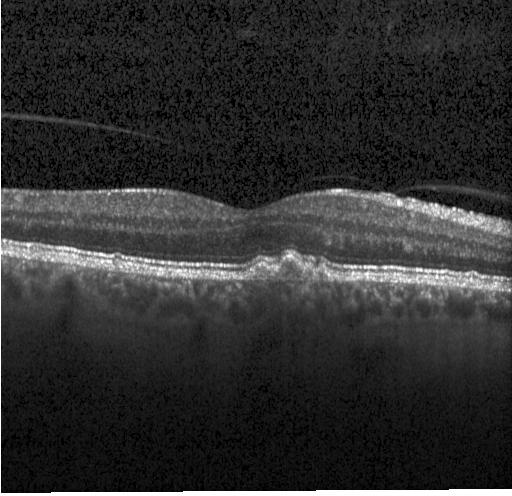 Centered on the fovea; instrument: Heidelberg Spectralis; retinal OCT cross-section.
Assessment: drusen.